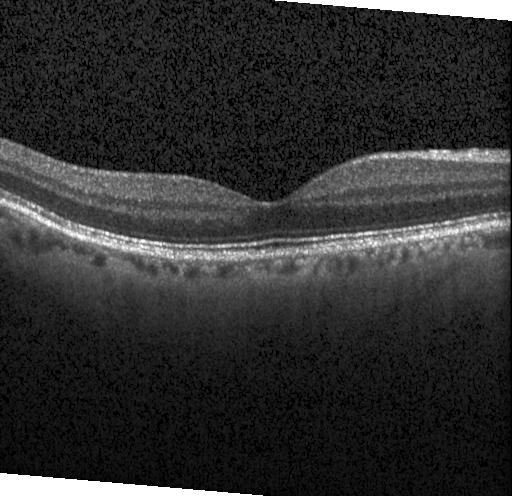

OCT scan showing no evidence of choroidal neovascularization, diabetic macular edema, or drusen.